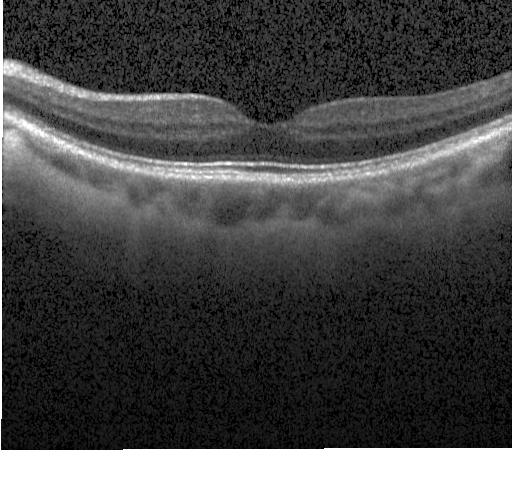
The scan shows no choroidal neovascularization, diabetic macular edema, or drusen.